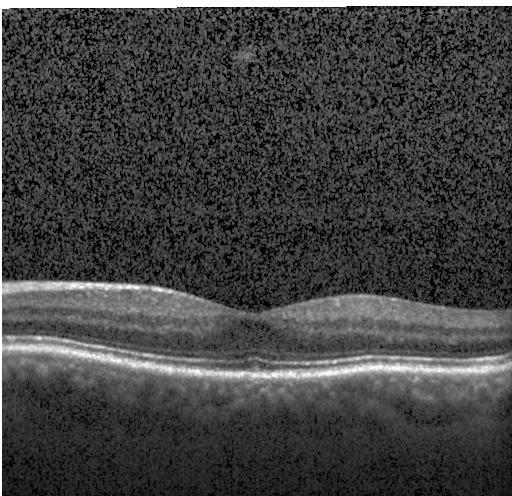

Macular OCT: neither choroidal neovascularization, diabetic macular edema, nor drusen.